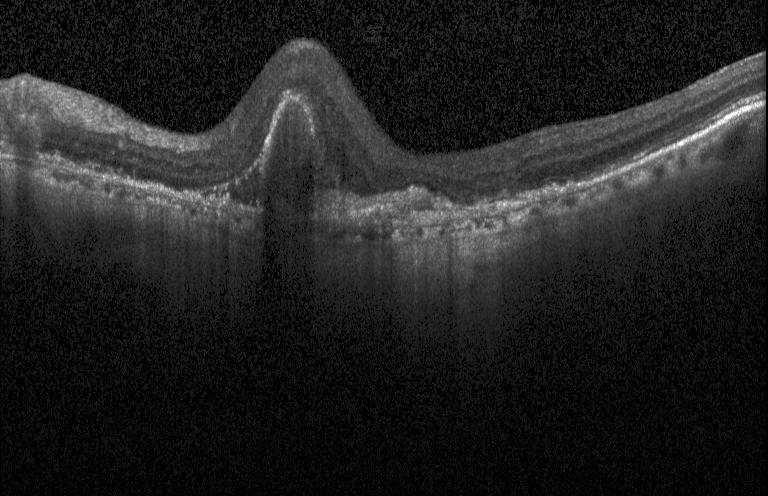 A choroidal neovascular membrane.